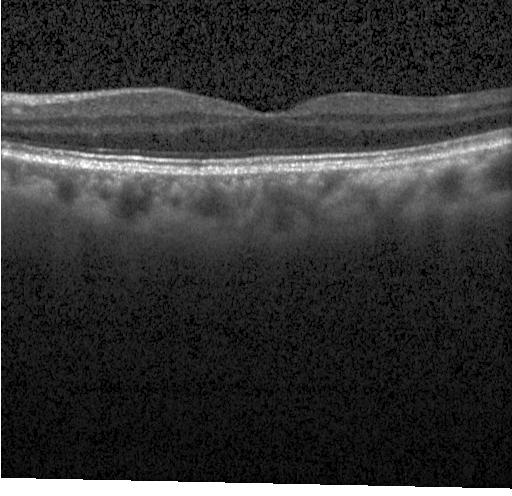

Diagnosis: neither CNV, DME, nor drusen.